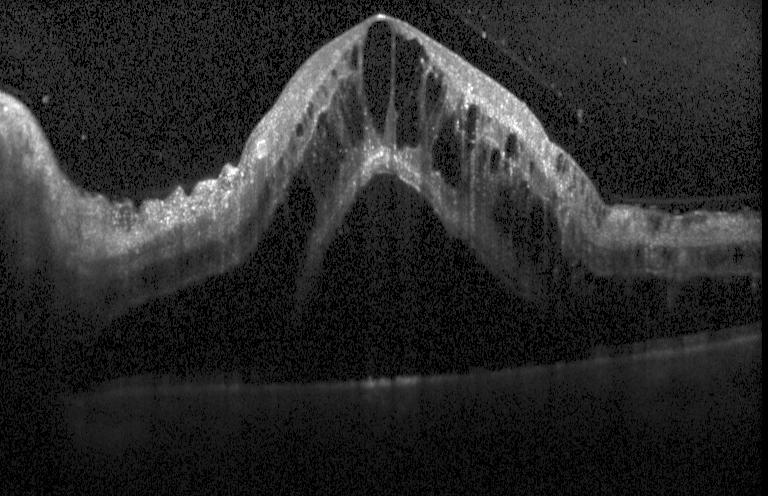 Retinal OCT B-scan — Finding: diabetic macular edema.